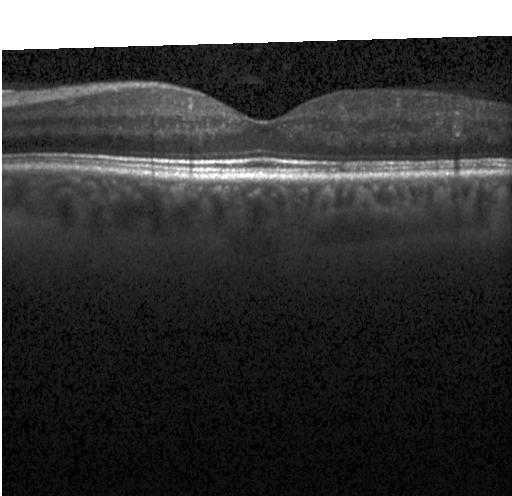
Heidelberg Spectralis OCT system; SD-OCT; fovea-centered; retinal OCT cross-section.
Impression: no choroidal neovascularization, diabetic macular edema, or drusen.